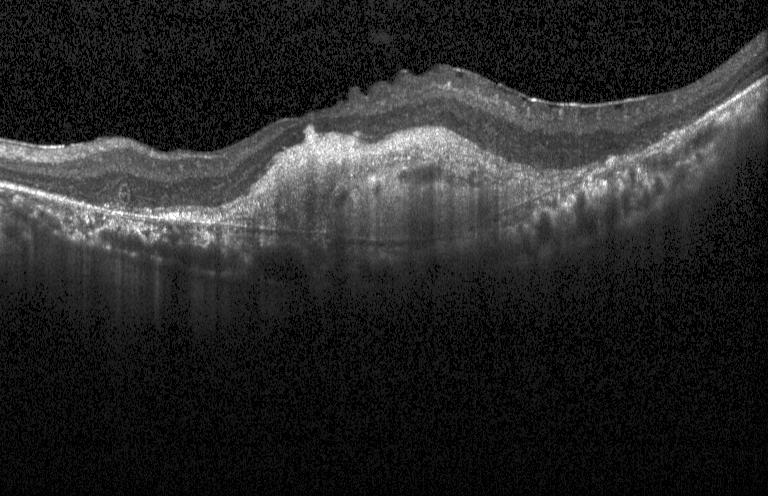

Finding: a choroidal neovascular membrane.